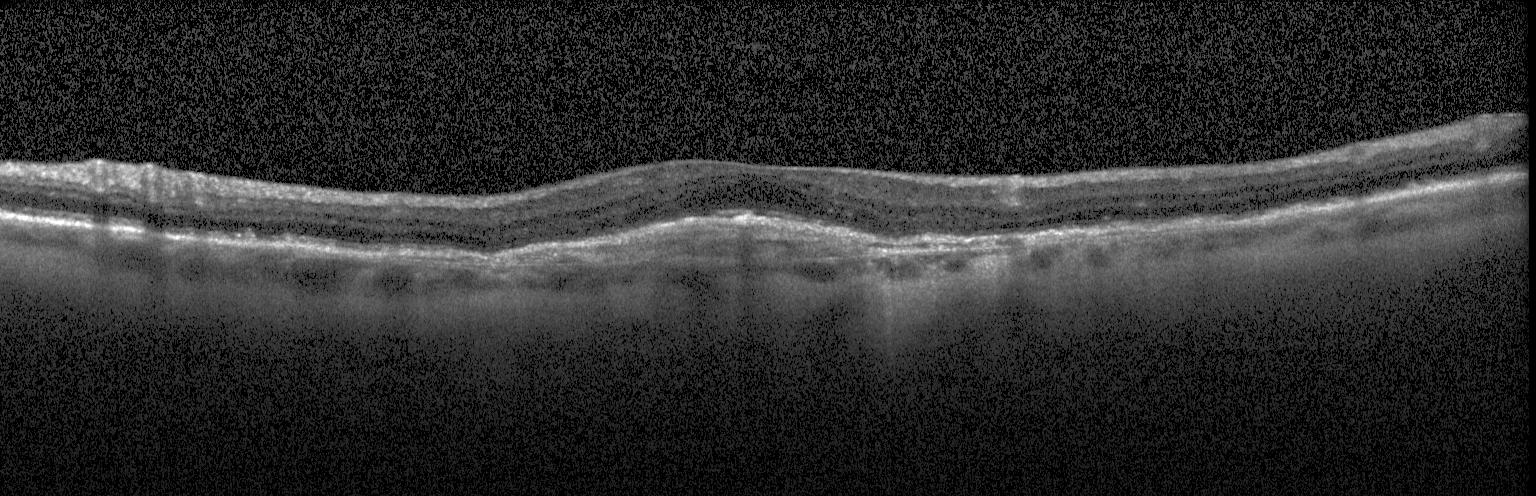
Spectral-domain OCT B-scan: a choroidal neovascular membrane.